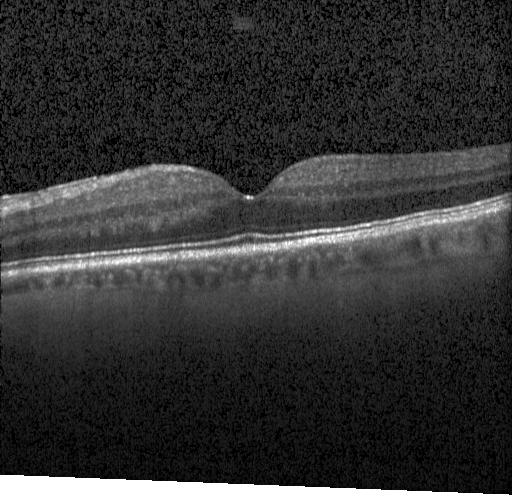
OCT B-scan.
The scan shows no choroidal neovascularization, diabetic macular edema, or drusen.